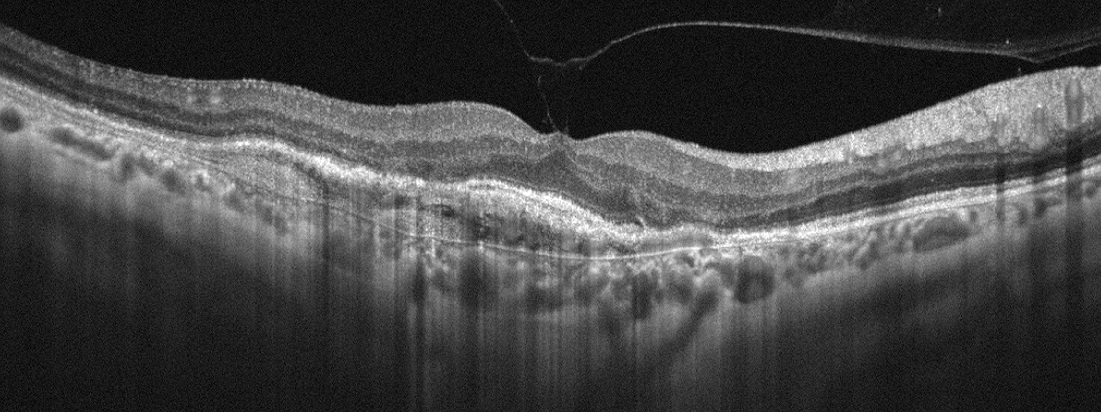
Optical coherence tomography B-scan — Finding: age-related macular degeneration.